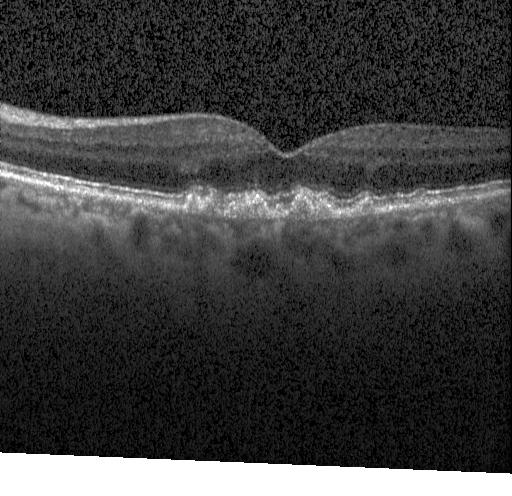 Optical coherence tomography scan; SD-OCT; horizontal scan through the fovea. Finding: sub-RPE drusenoid deposits.